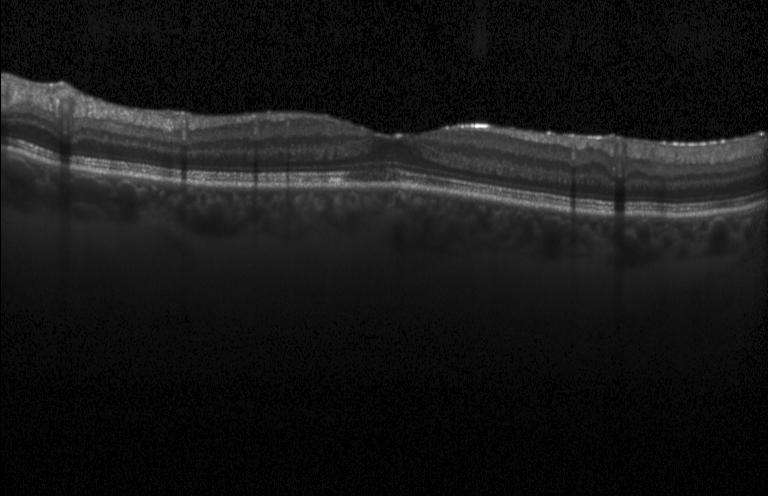

Impression: no choroidal neovascularization, no diabetic macular edema, and no drusen.